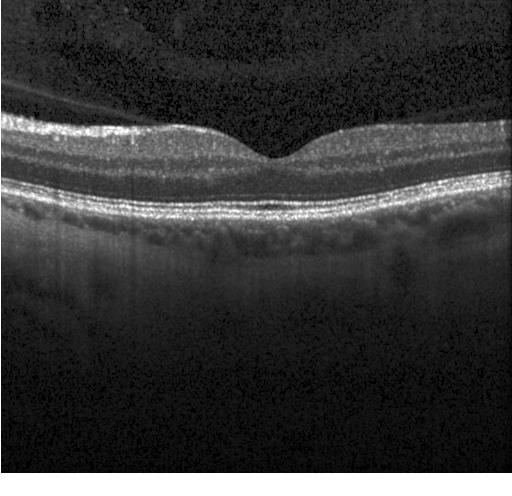 Finding: no evidence of choroidal neovascularization, diabetic macular edema, or drusen.